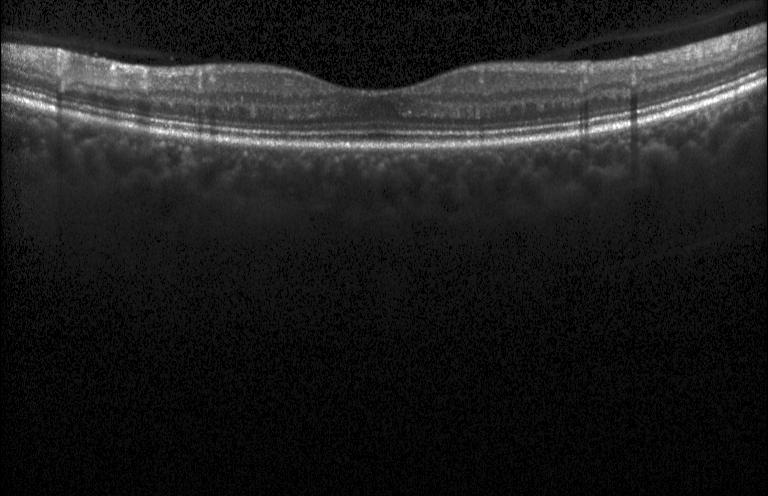
Retinal OCT cross-section.
Finding: no choroidal neovascularization, no diabetic macular edema, and no drusen.